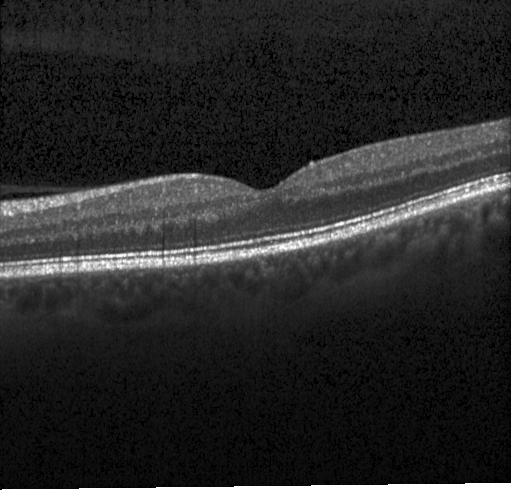 Impression: no CNV, DME, or drusen.